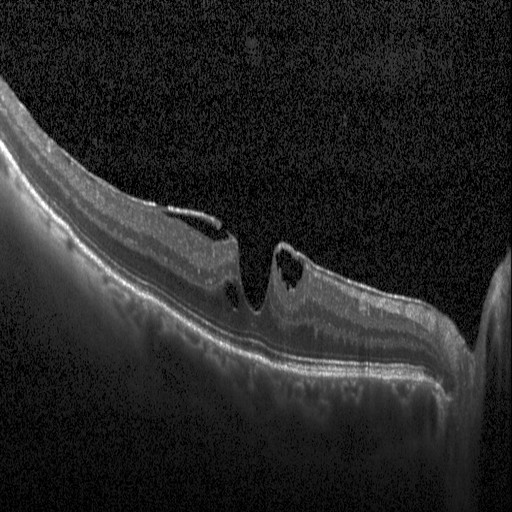
Instrument: Heidelberg Spectralis; retinal OCT cross-section; spectral-domain OCT; horizontal scan through the fovea.
This B-scan demonstrates DME.